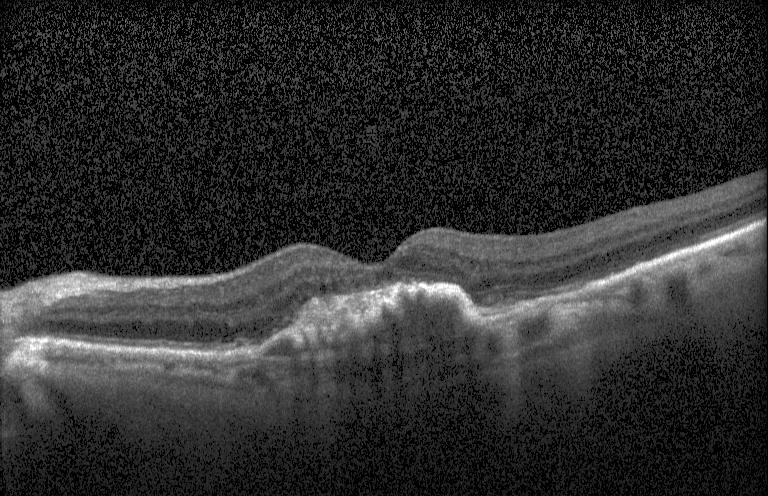

Retinal OCT cross-section; Heidelberg Spectralis; centered on the fovea; spectral-domain OCT — Impression: CNV.